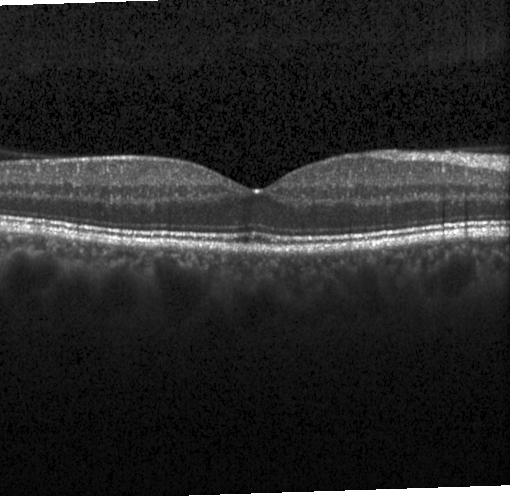
OCT finding: no choroidal neovascularization, diabetic macular edema, or drusen.